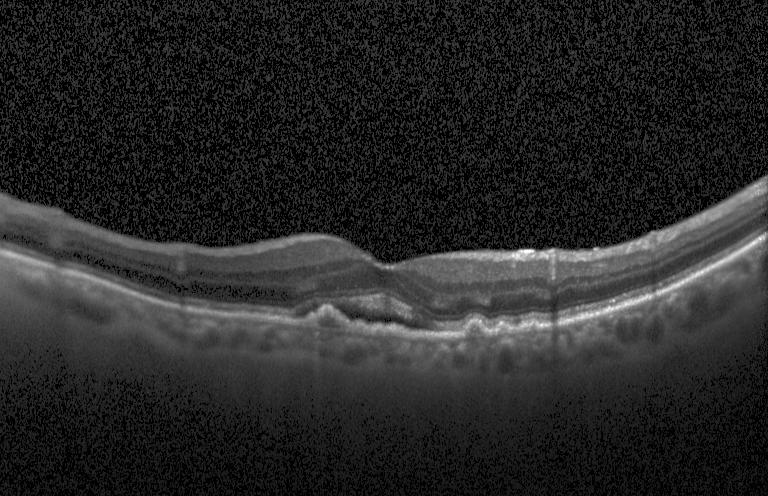
The scan shows CNV.